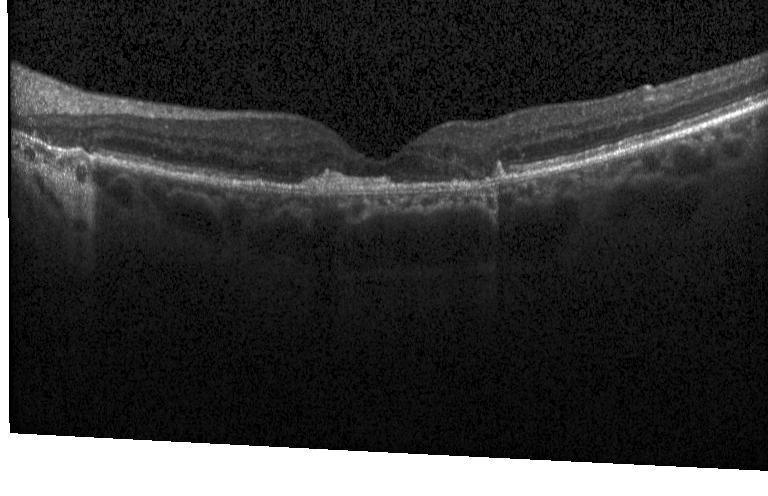 Retinal OCT cross-section.
OCT finding: a choroidal neovascular membrane.